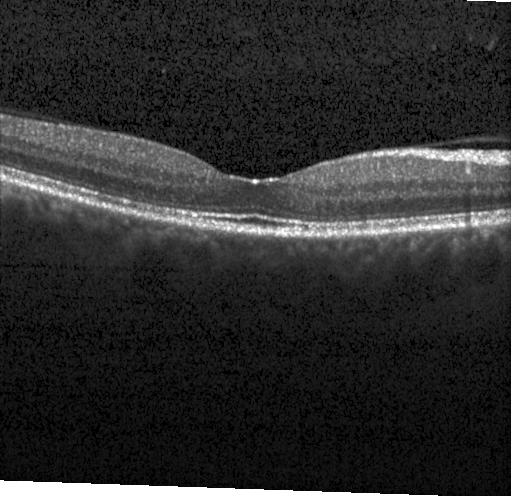

Heidelberg Spectralis OCT system, spectral-domain optical coherence tomography, OCT line scan. Macular OCT: no evidence of CNV, DME, or drusen.